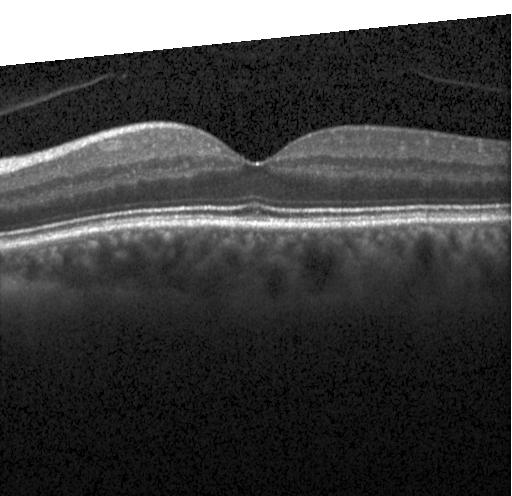
OCT scan showing no evidence of choroidal neovascularization, diabetic macular edema, or drusen.